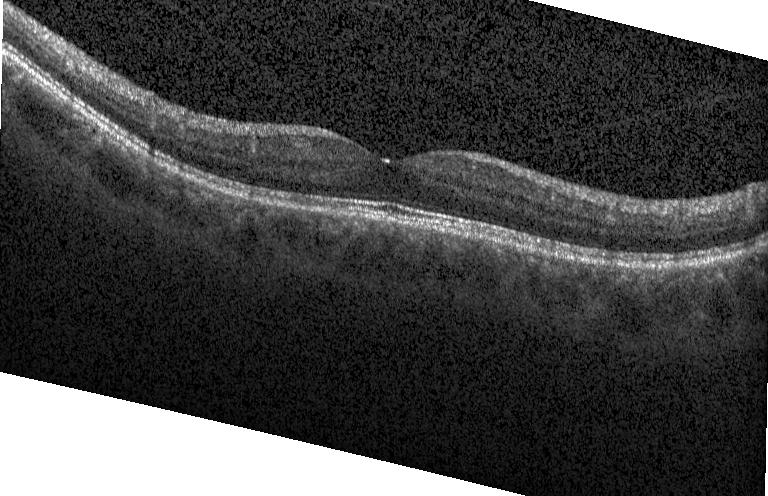
OCT B-scan, horizontal scan through the fovea — Assessment: neither choroidal neovascularization, diabetic macular edema, nor drusen.